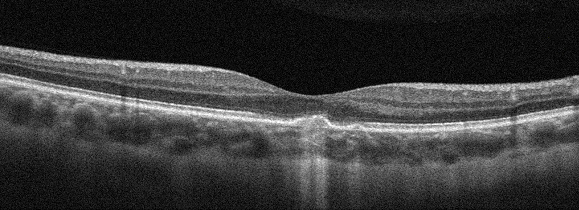
Retinal OCT B-scan; oculus sinister — Assessment: age-related macular degeneration (AMD).